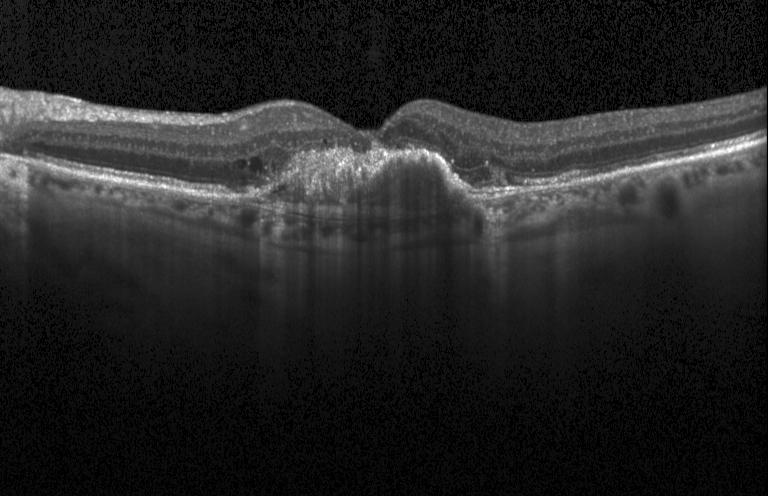
OCT finding: choroidal neovascularization (CNV).